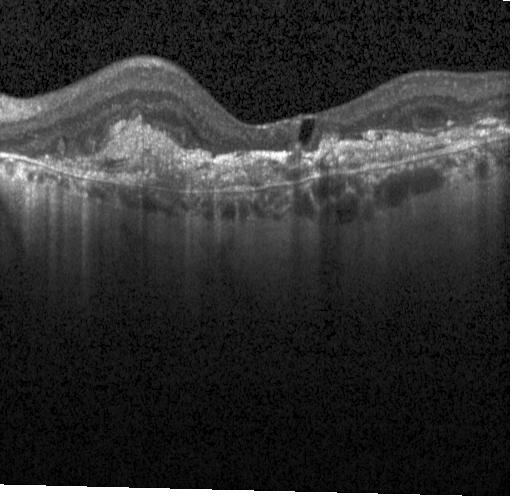
Finding: a choroidal neovascular membrane.